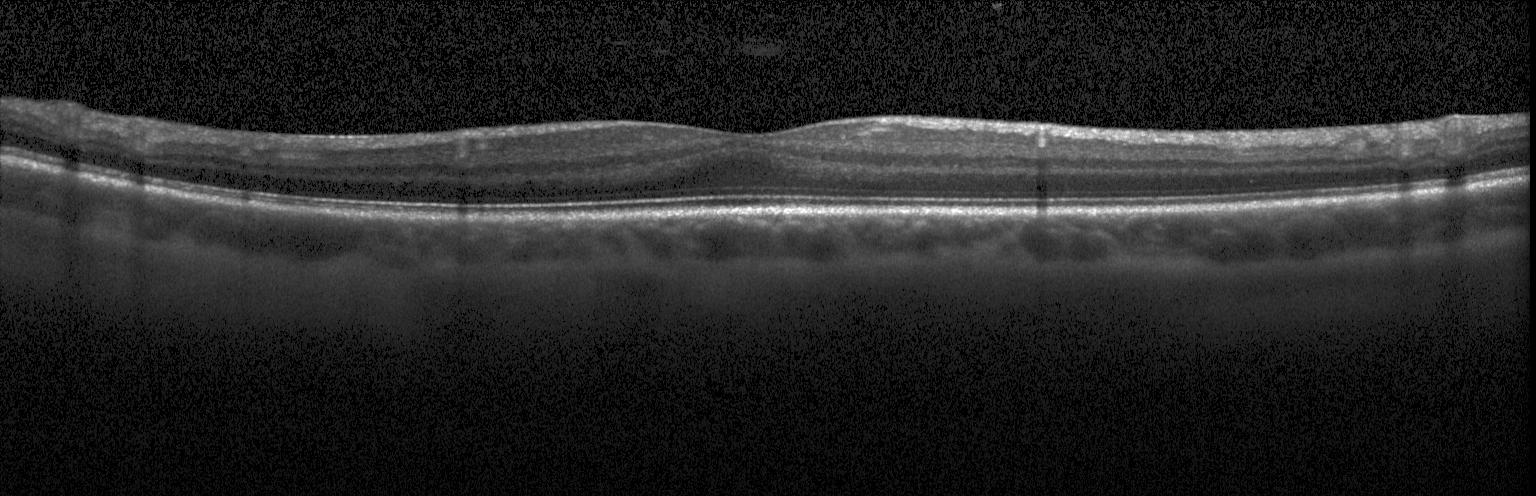
Instrument: Heidelberg Spectralis; OCT B-scan.
No CNV, no DME, and no drusen.